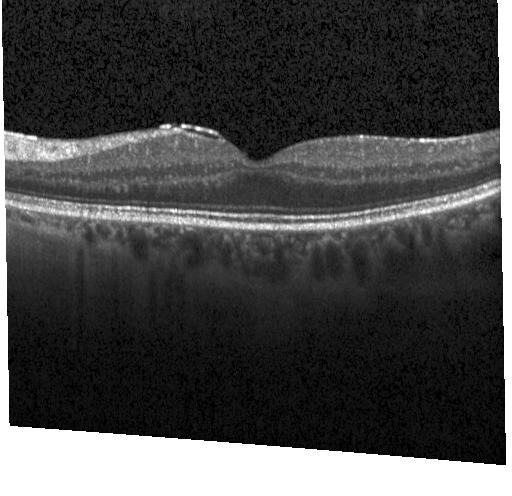

Diagnosis: neither choroidal neovascularization, diabetic macular edema, nor drusen.